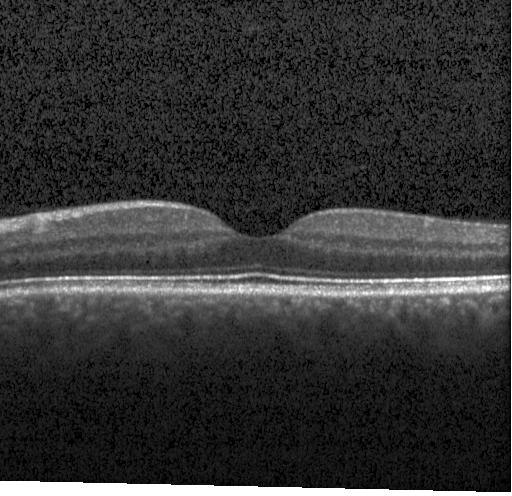 Retinal OCT B-scan; spectral-domain optical coherence tomography — This B-scan demonstrates no evidence of CNV, DME, or drusen.